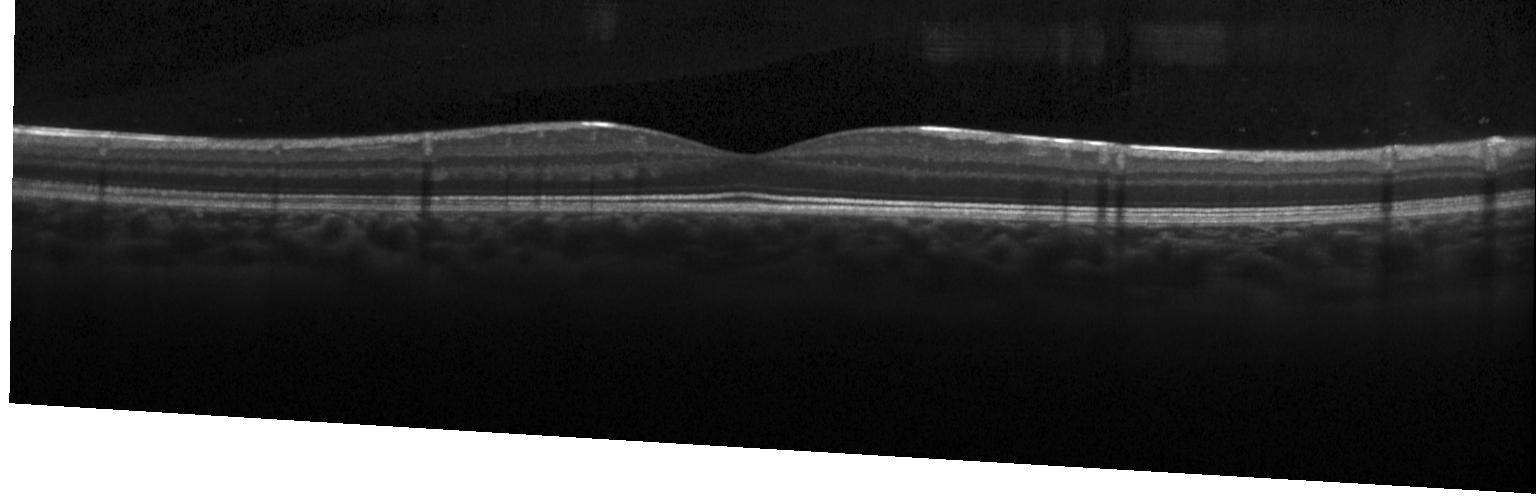
Neither choroidal neovascularization, diabetic macular edema, nor drusen.